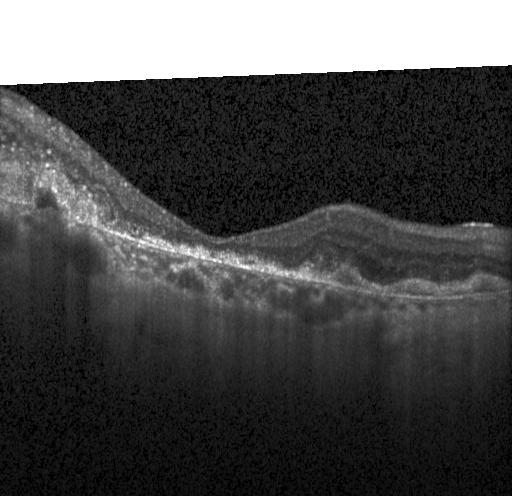 Impression: a choroidal neovascular membrane.